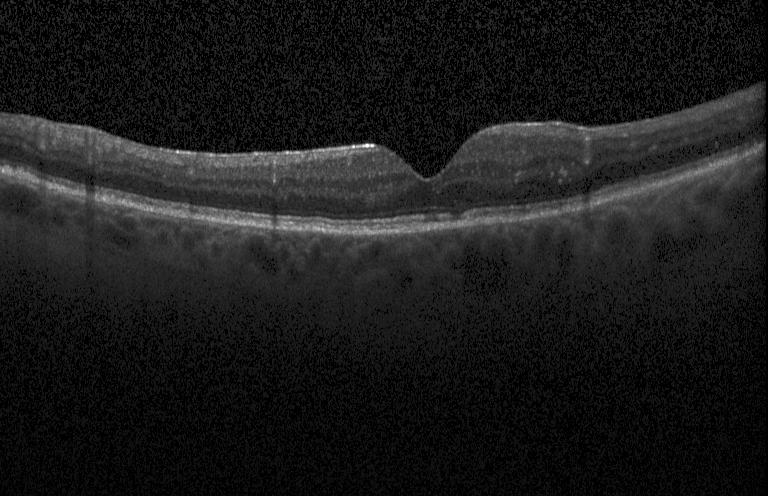
Retinal OCT cross-section. Centered on the fovea. Spectral-domain OCT.
Diagnosis: no evidence of CNV, DME, or drusen.